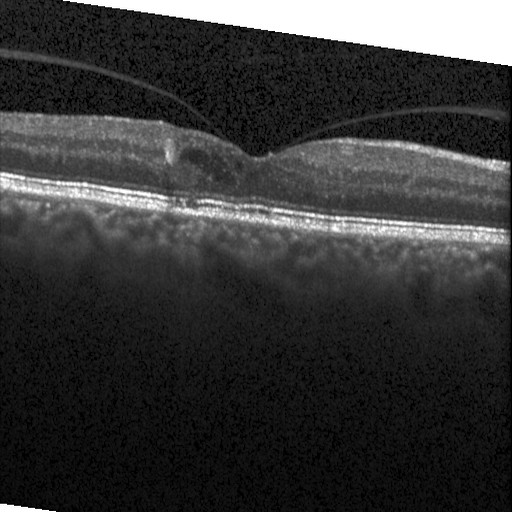

OCT line scan.
DME.